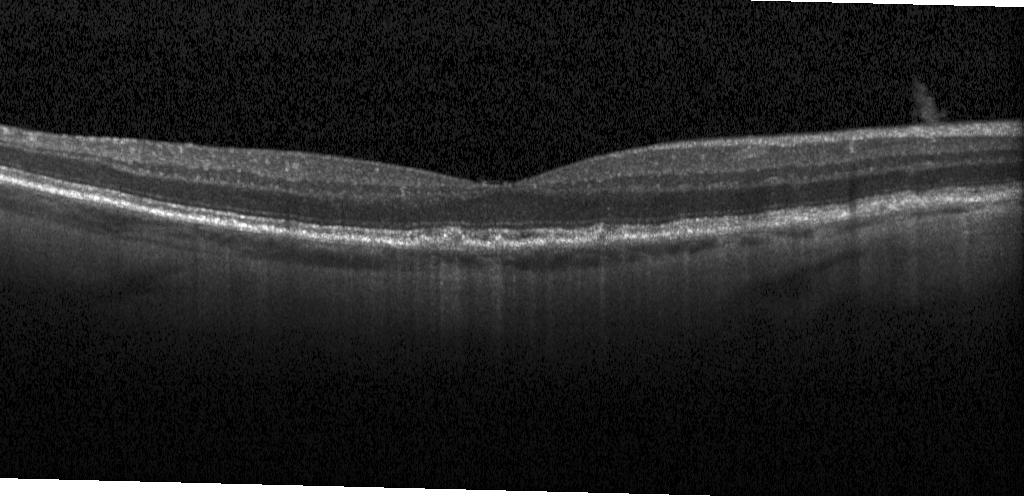 Retinal OCT cross-section showing multiple drusen.